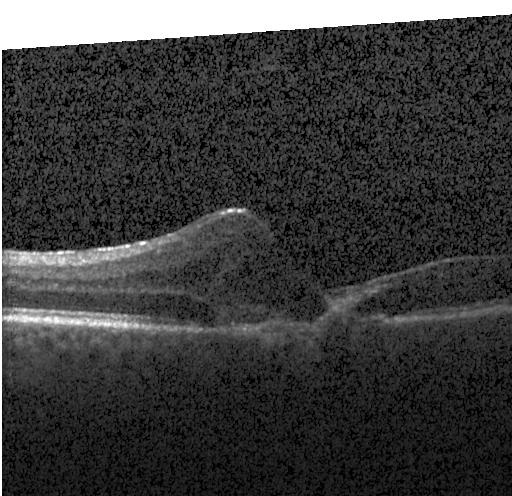

Acquired on a Heidelberg Spectralis · macular scan · OCT B-scan
Diagnosis: a choroidal neovascular membrane.